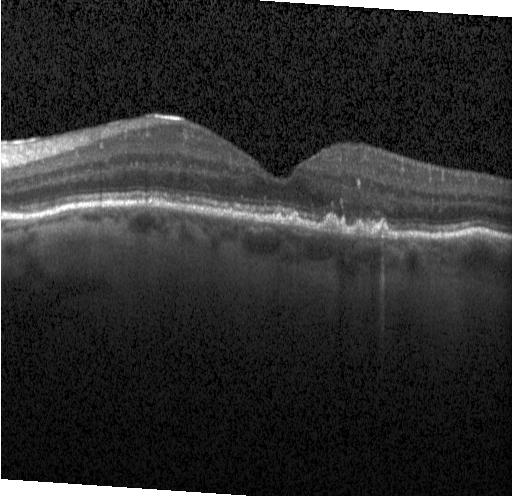

Spectral-domain optical coherence tomography, retinal OCT cross-section, acquired on a Heidelberg Spectralis, through the macula — This B-scan demonstrates sub-RPE drusenoid deposits.